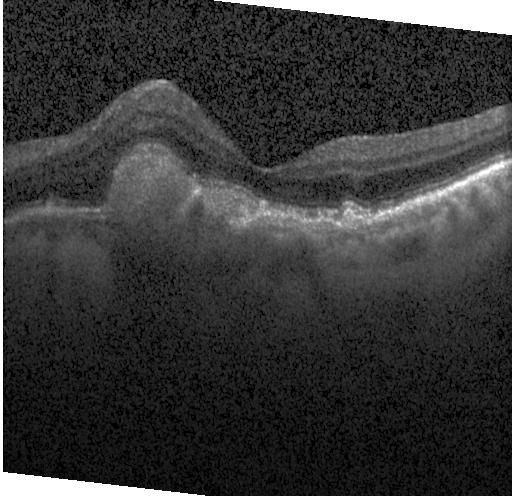

Impression: choroidal neovascularization (CNV).